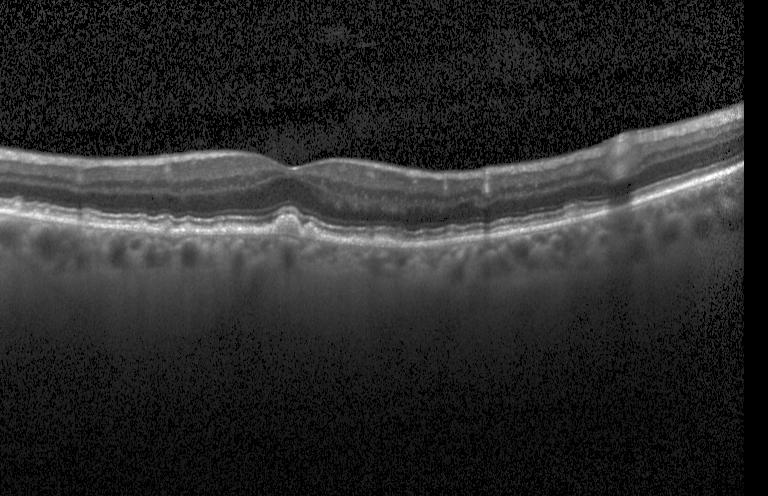
The scan shows multiple drusen.